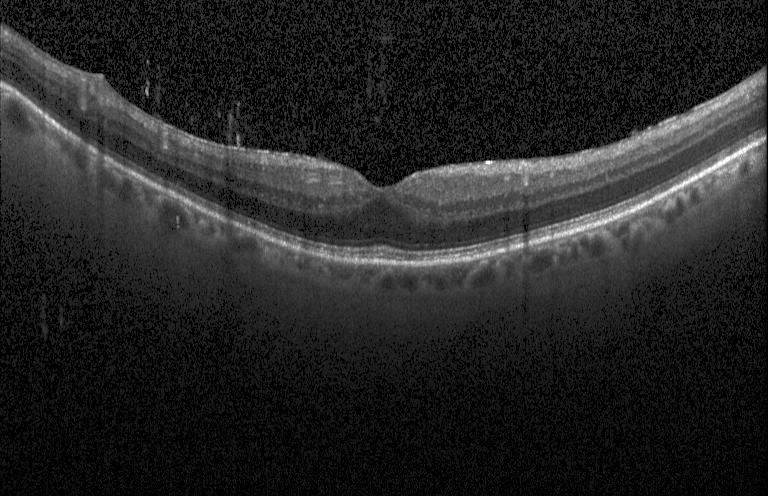
Impression: no choroidal neovascularization, no diabetic macular edema, and no drusen.